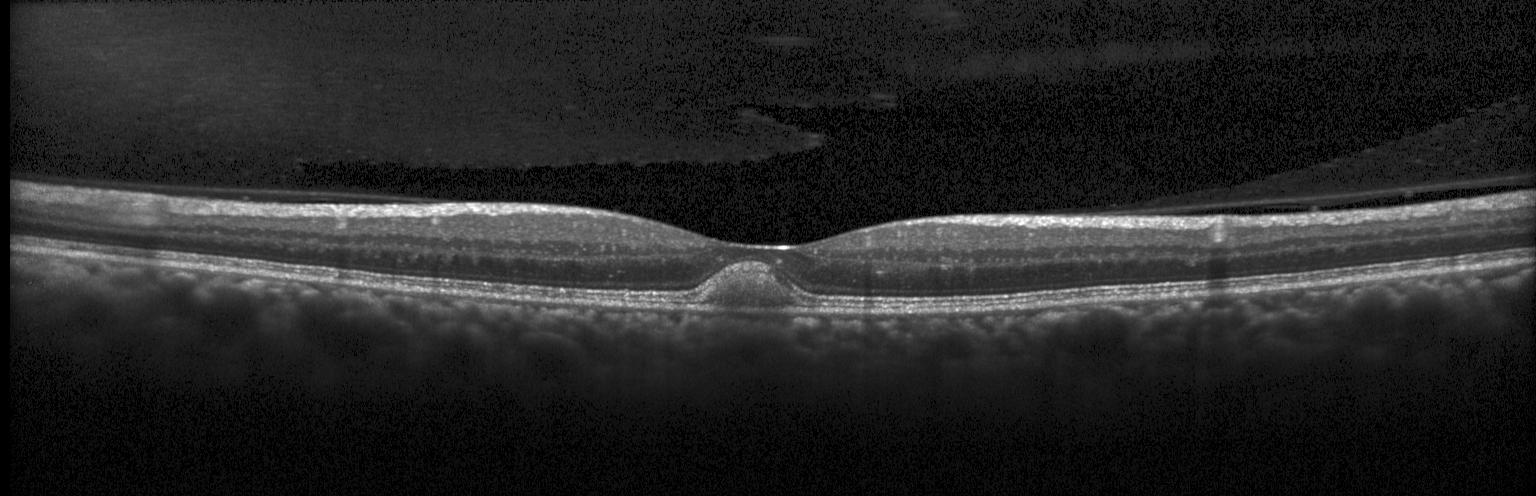 Finding: choroidal neovascularization (CNV).